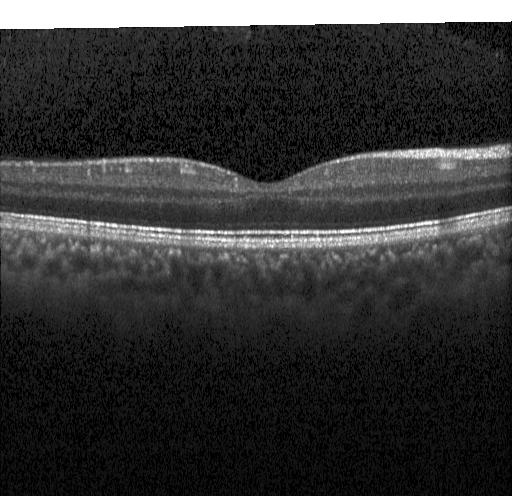 Diagnosis: no choroidal neovascularization, no diabetic macular edema, and no drusen.